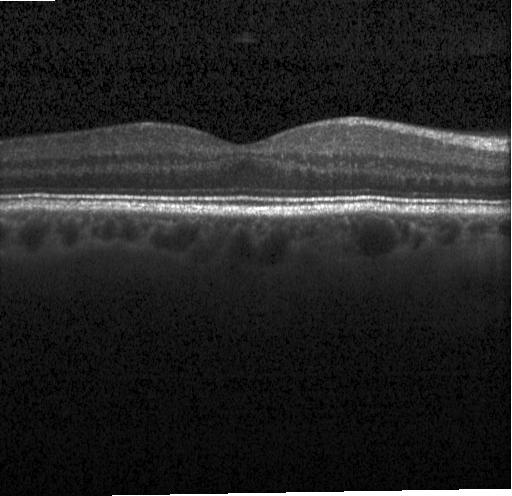

Dx: neither choroidal neovascularization, diabetic macular edema, nor drusen.